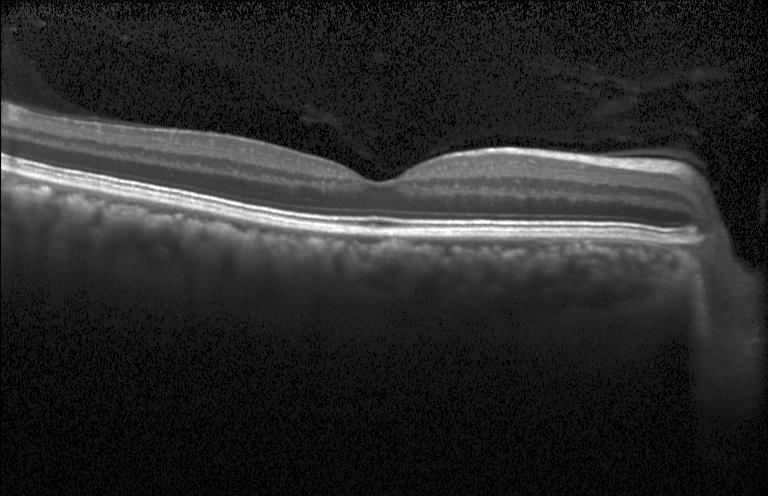 No CNV, DME, or drusen.